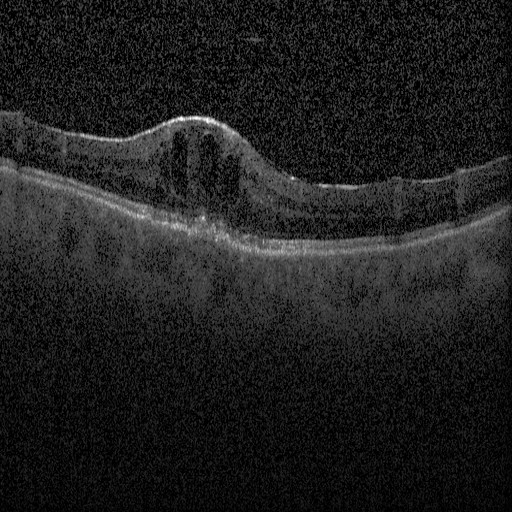 Retinal OCT B-scan
This B-scan demonstrates diabetic macular edema (DME).